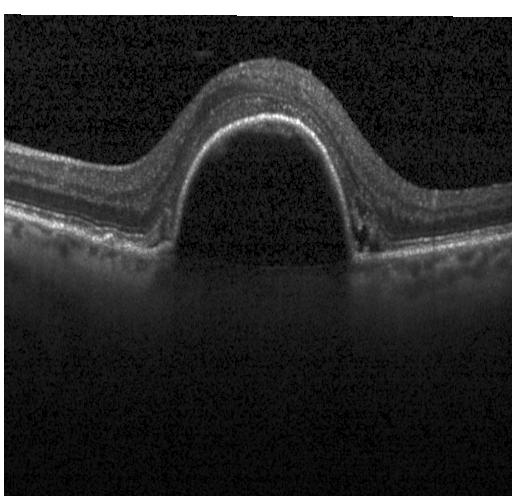

Heidelberg Spectralis; optical coherence tomography B-scan.
Finding: choroidal neovascularization (CNV).